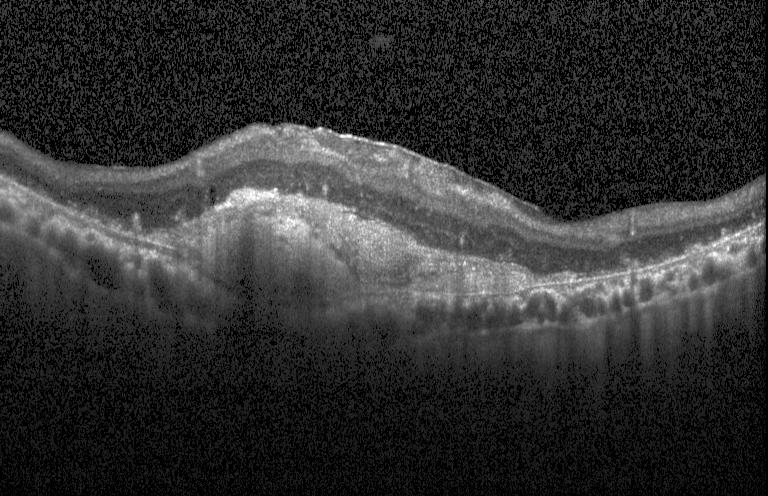

Impression: CNV.